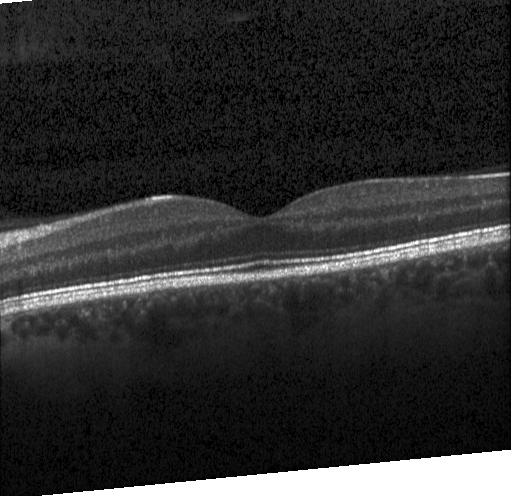 OCT line scan.
Finding: neither choroidal neovascularization, diabetic macular edema, nor drusen.